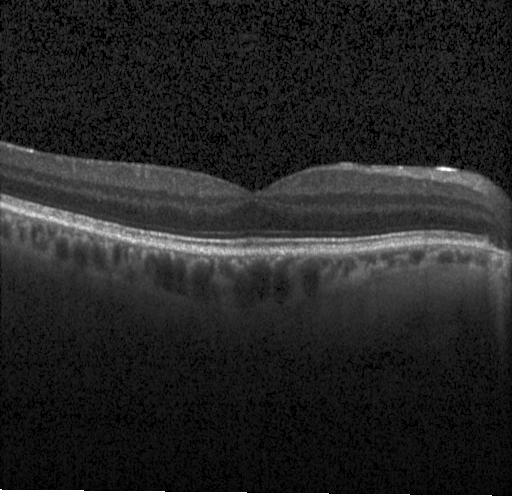
Retinal OCT B-scan. Finding: no CNV, no DME, and no drusen.